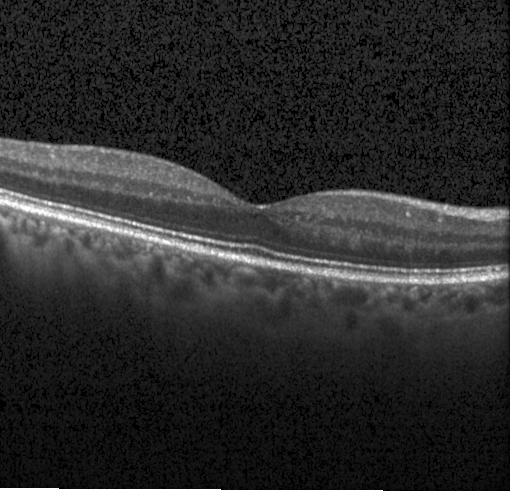
Spectral-domain optical coherence tomography, Heidelberg Spectralis, OCT B-scan, fovea-centered
Macular OCT: no evidence of CNV, DME, or drusen.